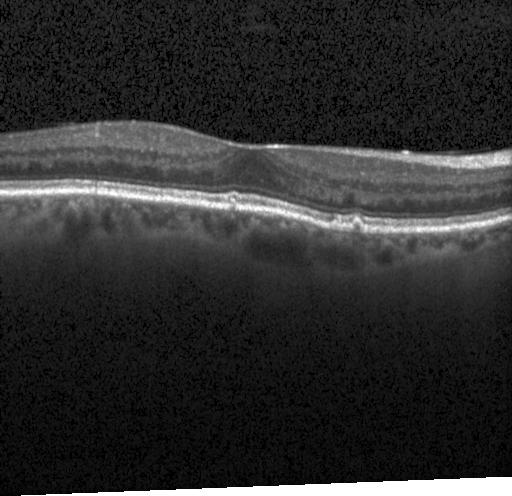

Centered on the fovea, SD-OCT, instrument: Heidelberg Spectralis, retinal OCT cross-section
This B-scan demonstrates multiple drusen.